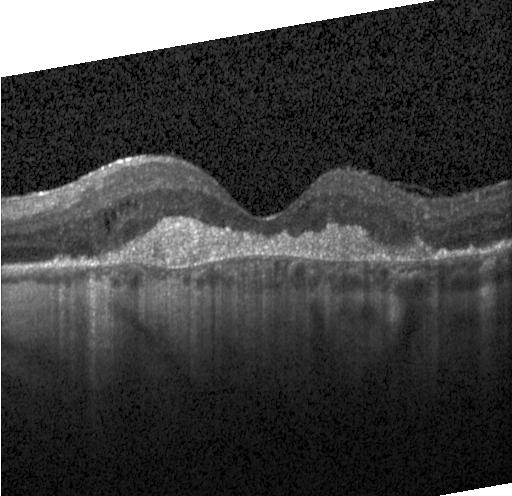

Centered on the fovea. Retinal OCT B-scan
Diagnosis: a choroidal neovascular membrane.